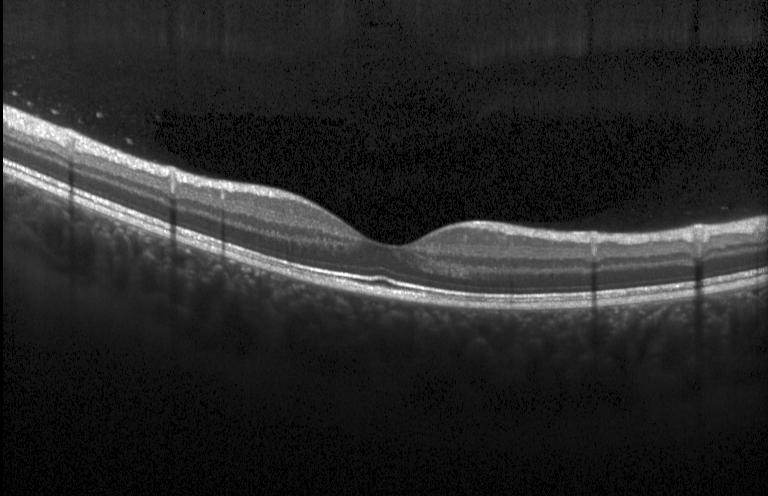
OCT B-scan.
OCT finding: neither choroidal neovascularization, diabetic macular edema, nor drusen.